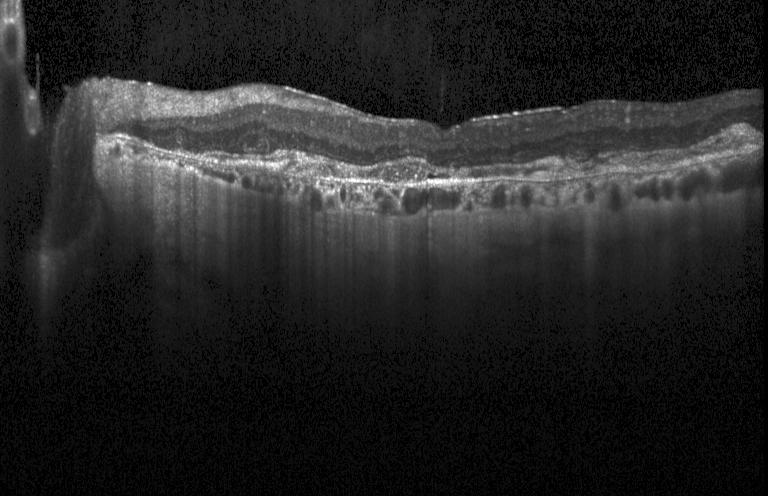
CNV.